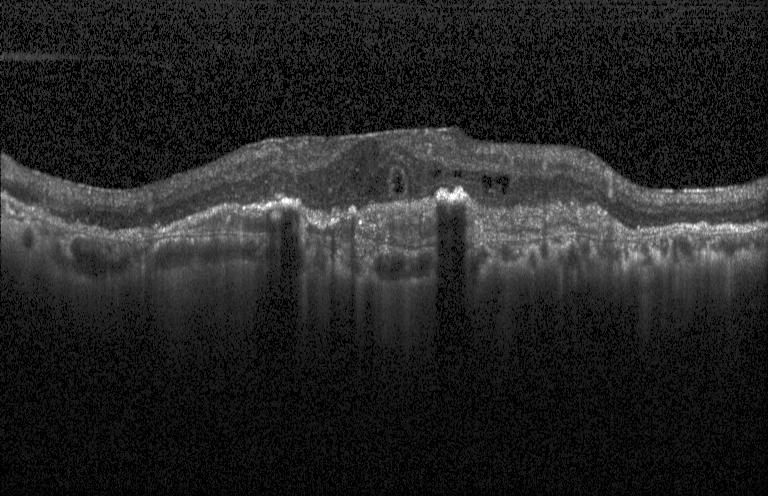 Heidelberg Spectralis, fovea-centered, optical coherence tomography scan, spectral-domain OCT.
Impression: a choroidal neovascular membrane.